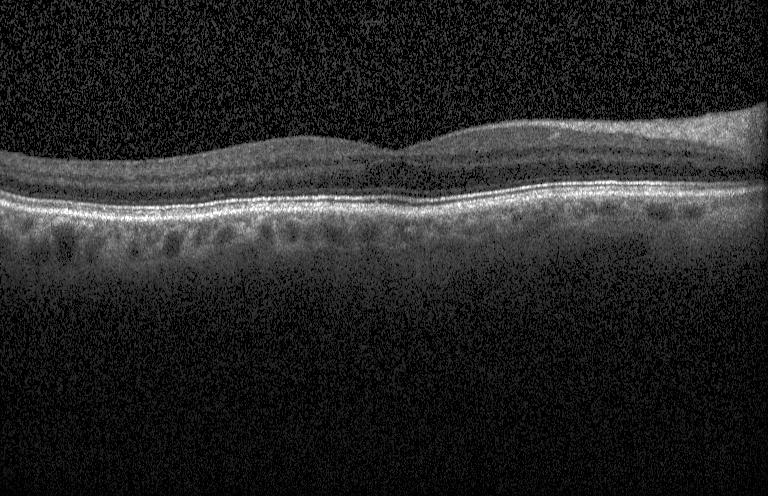 Acquired on a Heidelberg Spectralis. OCT line scan. Through the macula.
Assessment: no evidence of choroidal neovascularization, diabetic macular edema, or drusen.